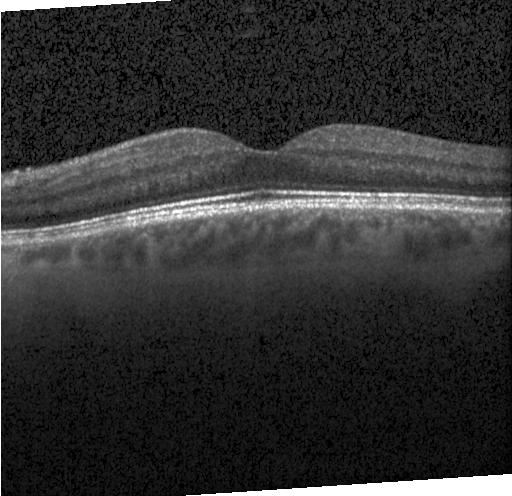
Macular OCT: neither CNV, DME, nor drusen.